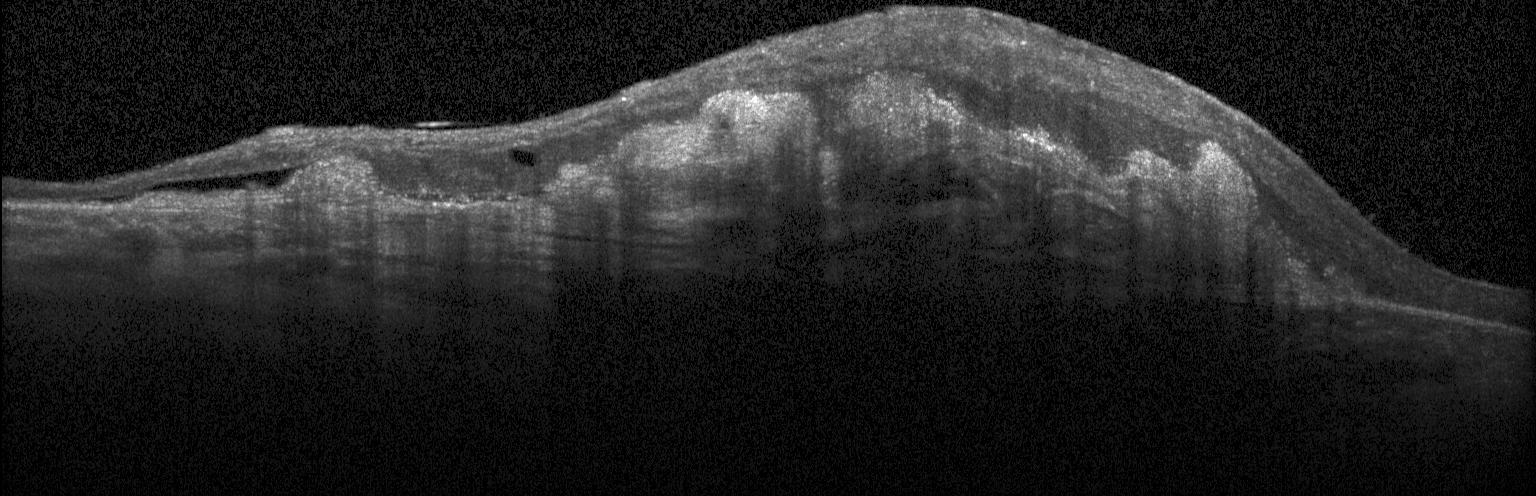
A choroidal neovascular membrane.